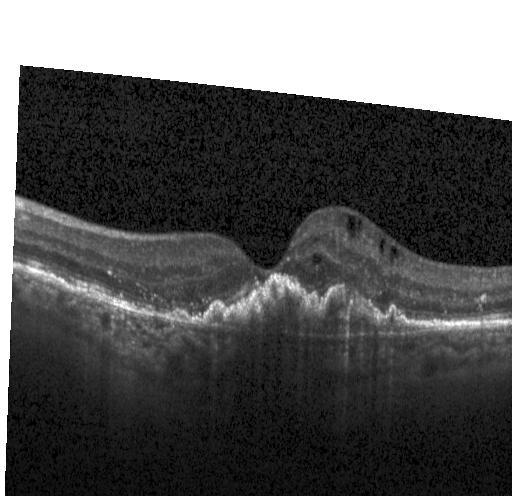
This B-scan demonstrates choroidal neovascularization.